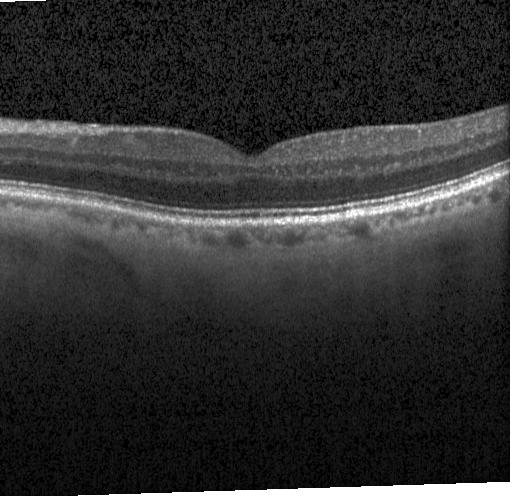

Finding: neither choroidal neovascularization, diabetic macular edema, nor drusen.